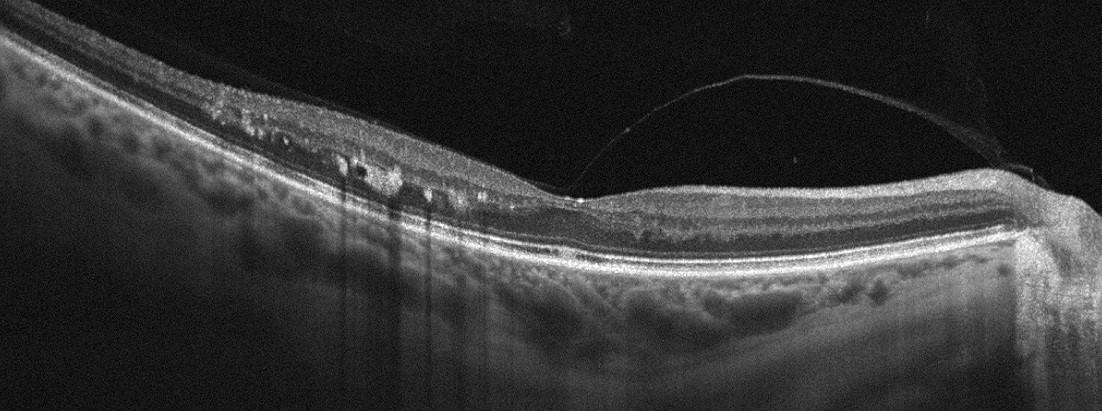

Impression: diabetic macular edema (DME).